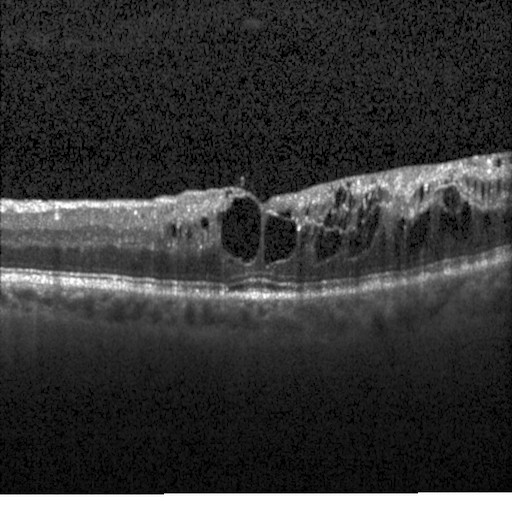
Heidelberg Spectralis · fovea-centered · retinal OCT cross-section. Assessment: diabetic macular edema (DME).